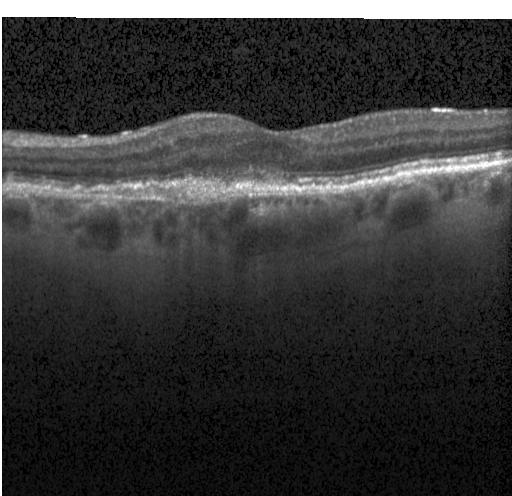
SD-OCT, acquired on a Heidelberg Spectralis, centered on the fovea, optical coherence tomography B-scan. Finding: a choroidal neovascular membrane.